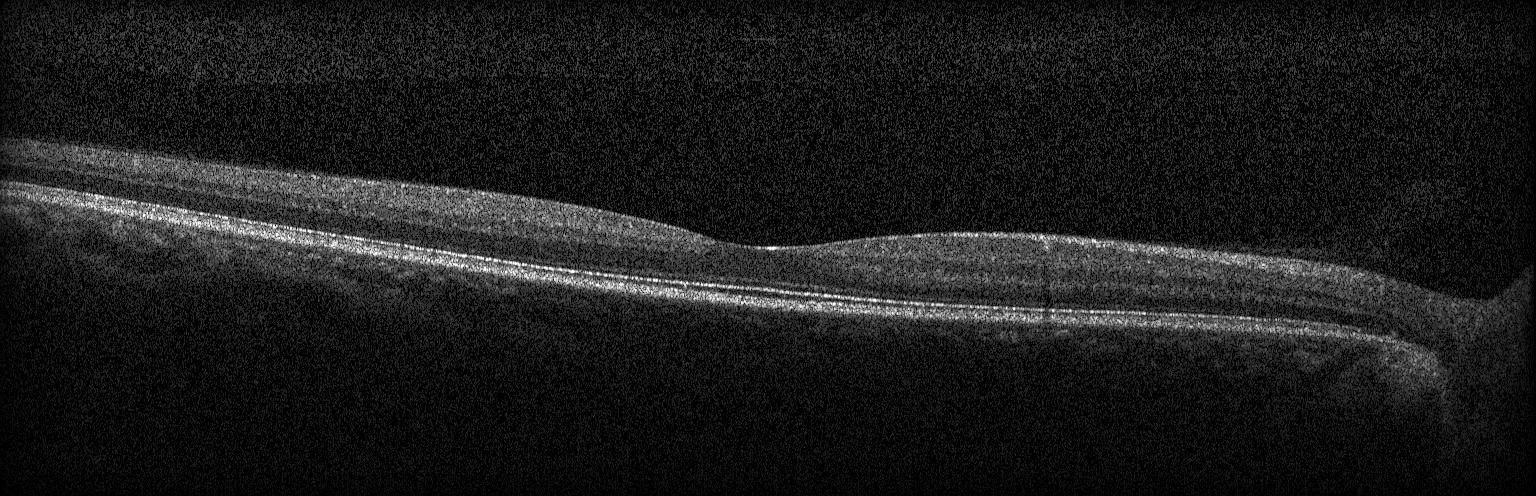 Spectral-domain OCT · acquired on a Heidelberg Spectralis · OCT B-scan · macular scan.
This B-scan demonstrates no choroidal neovascularization, no diabetic macular edema, and no drusen.